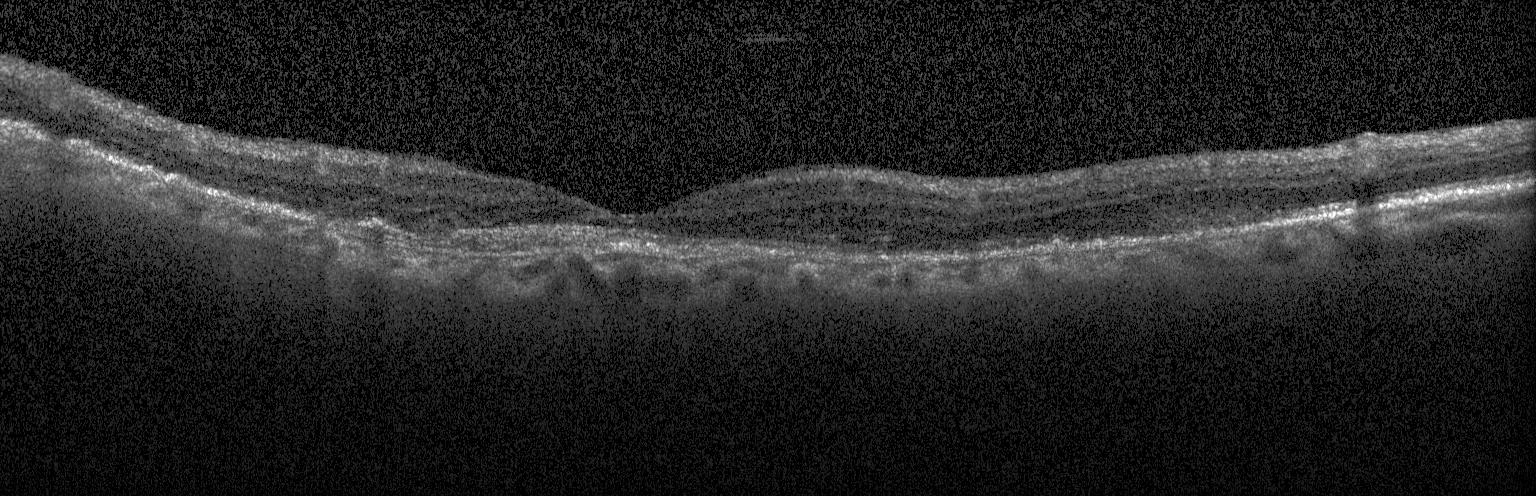
Fovea-centered. Spectral-domain optical coherence tomography. OCT B-scan. Heidelberg Spectralis OCT system
Assessment: a choroidal neovascular membrane.